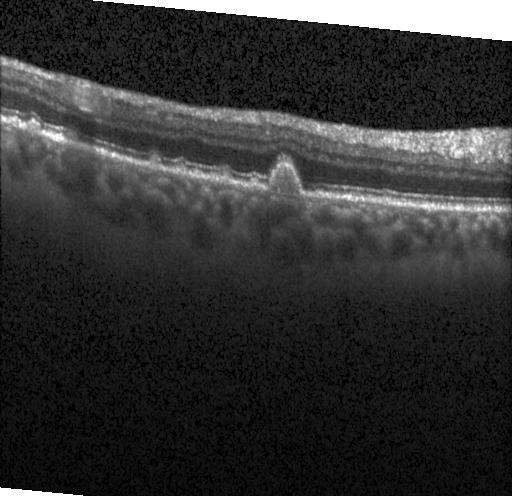

SD-OCT, acquired on a Heidelberg Spectralis, OCT B-scan. Diagnosis: drusen.